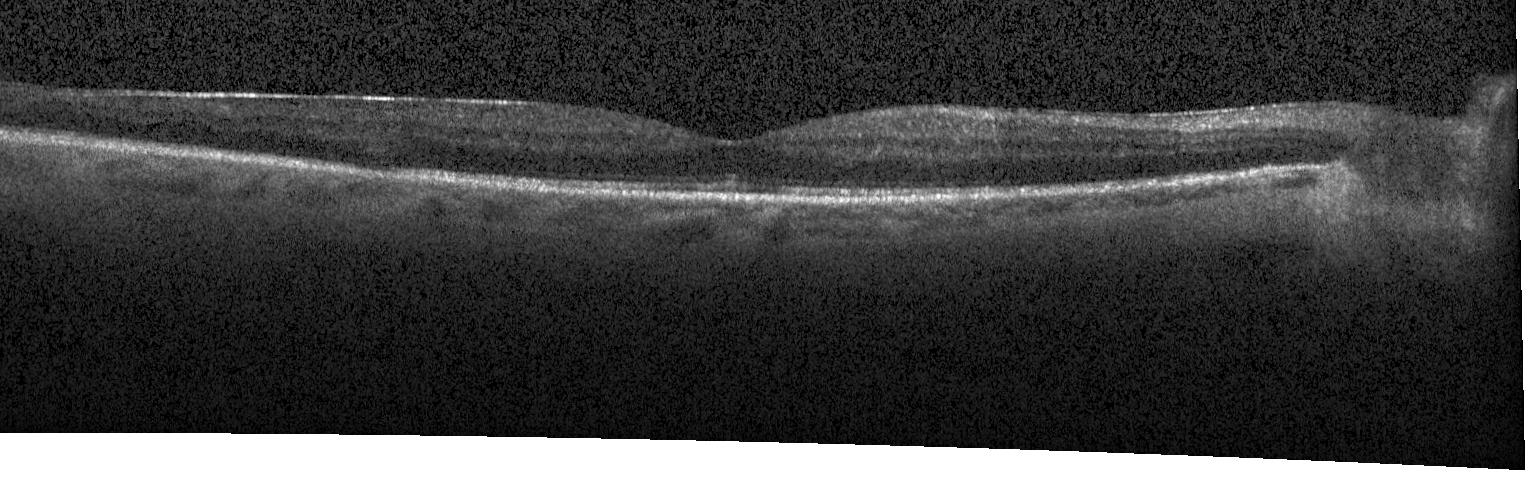
Retinal OCT B-scan · spectral-domain OCT. Finding: no evidence of CNV, DME, or drusen.